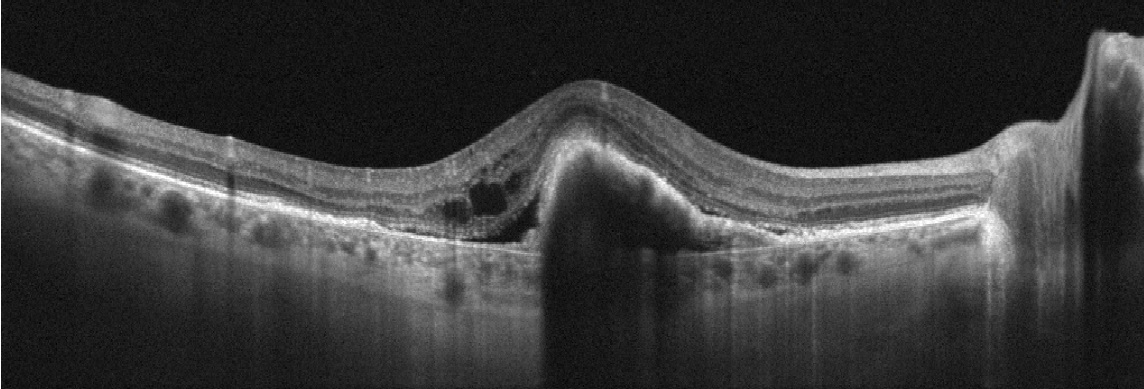

Instrument: Optovue Avanti RTVue XR · fovea-centered · optical coherence tomography scan.
Finding: AMD.